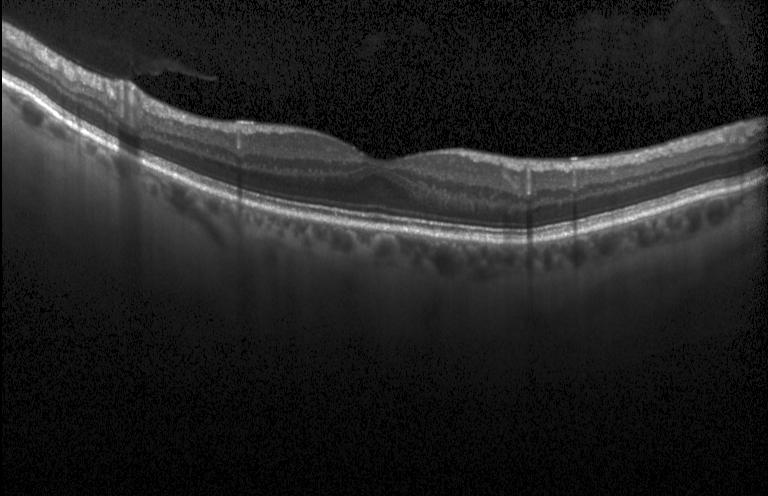

Heidelberg Spectralis OCT system. OCT B-scan. Centered on the fovea — Impression: no evidence of CNV, DME, or drusen.